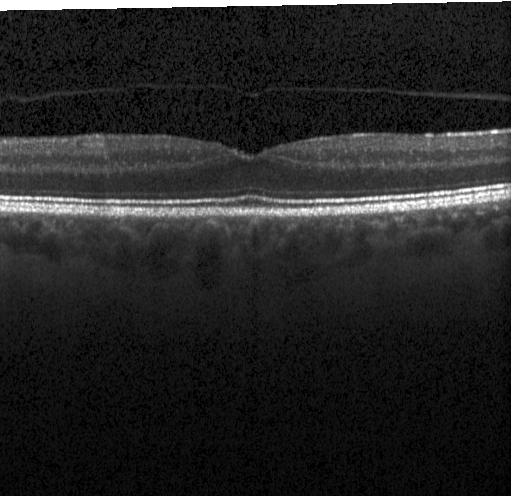 Instrument: Heidelberg Spectralis, centered on the fovea, spectral-domain optical coherence tomography, optical coherence tomography scan
Diagnosis: no choroidal neovascularization, diabetic macular edema, or drusen.